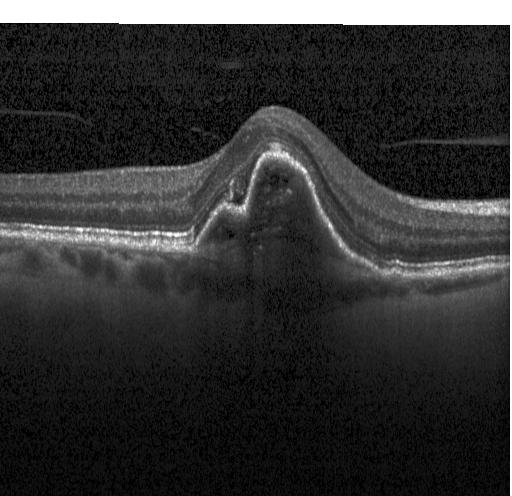

Retinal OCT cross-section, fovea-centered.
Impression: a choroidal neovascular membrane.